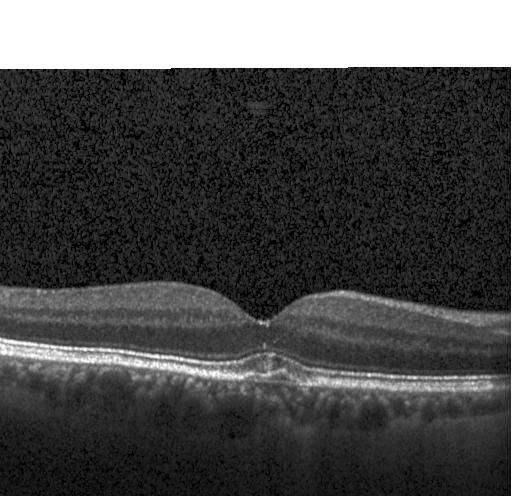

Spectral-domain optical coherence tomography, centered on the fovea, optical coherence tomography B-scan
Macular OCT: a choroidal neovascular membrane.